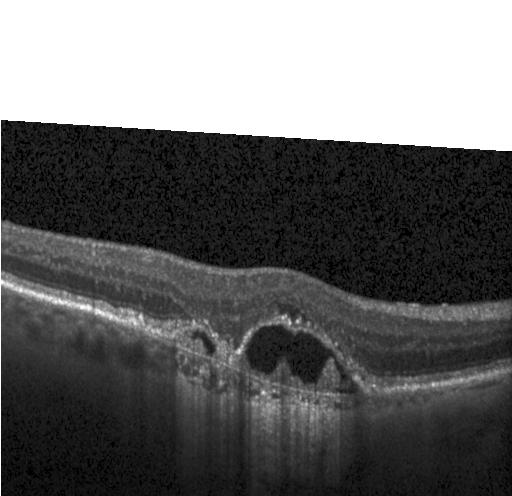
Impression: a choroidal neovascular membrane.